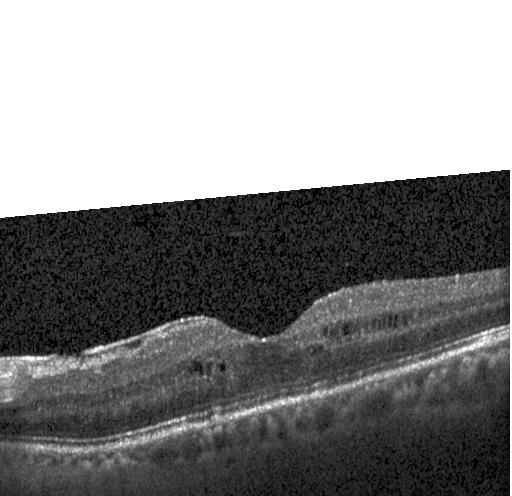

Optical coherence tomography B-scan, Heidelberg Spectralis, through the macula. Assessment: DME.